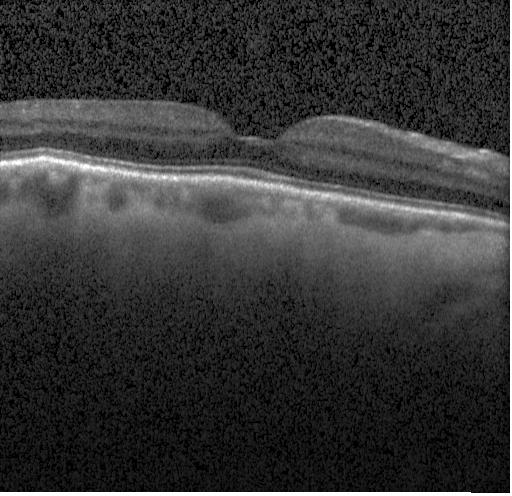 Acquired on a Heidelberg Spectralis; fovea-centered; spectral-domain optical coherence tomography; optical coherence tomography scan
The scan shows neither CNV, DME, nor drusen.